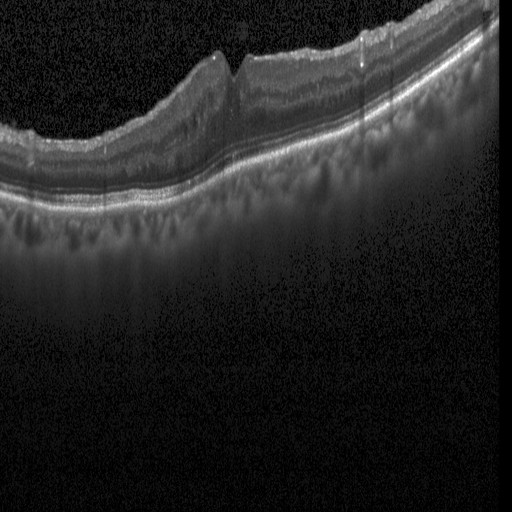
Finding: DME.